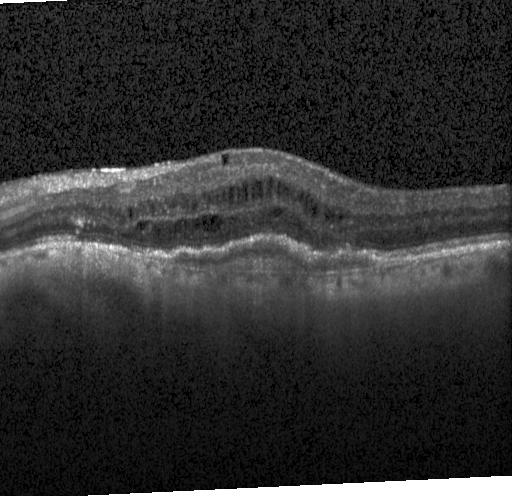

Retinal OCT B-scan. The scan shows a choroidal neovascular membrane.